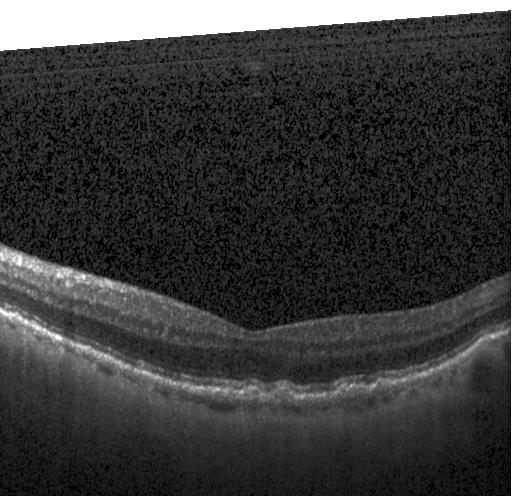
Heidelberg Spectralis. Optical coherence tomography B-scan. Finding: drusen.